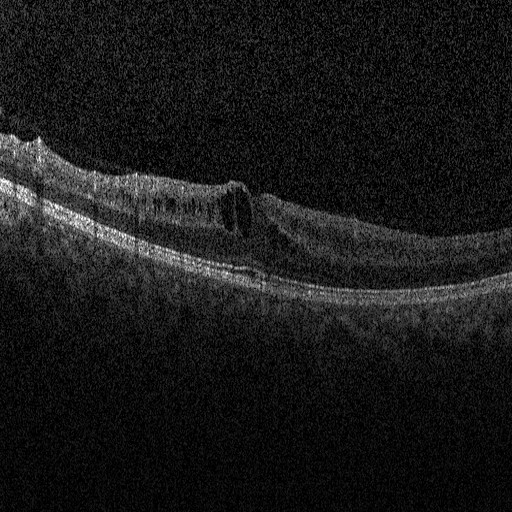

Diagnosis: diabetic macular edema (DME).